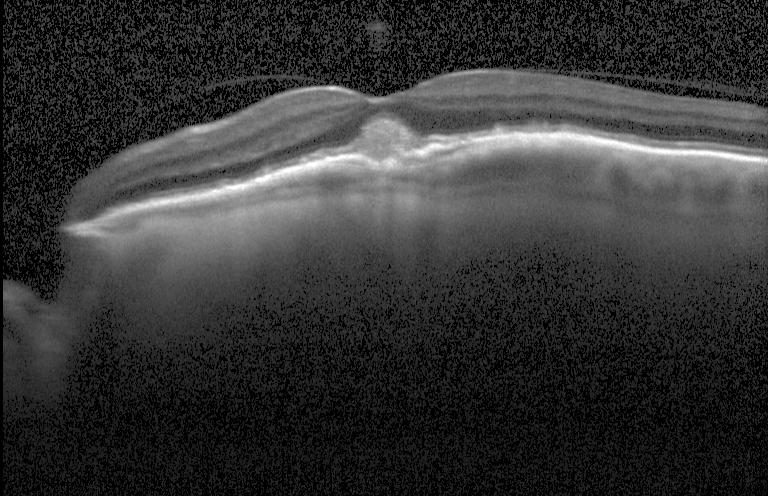

This B-scan demonstrates choroidal neovascularization.